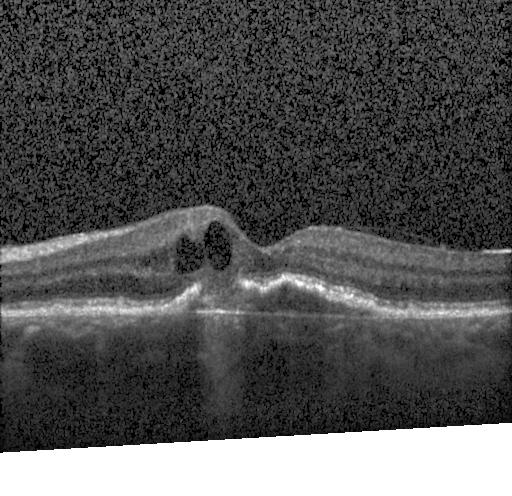

Acquired on a Heidelberg Spectralis. Retinal OCT B-scan. Macular OCT: choroidal neovascularization.